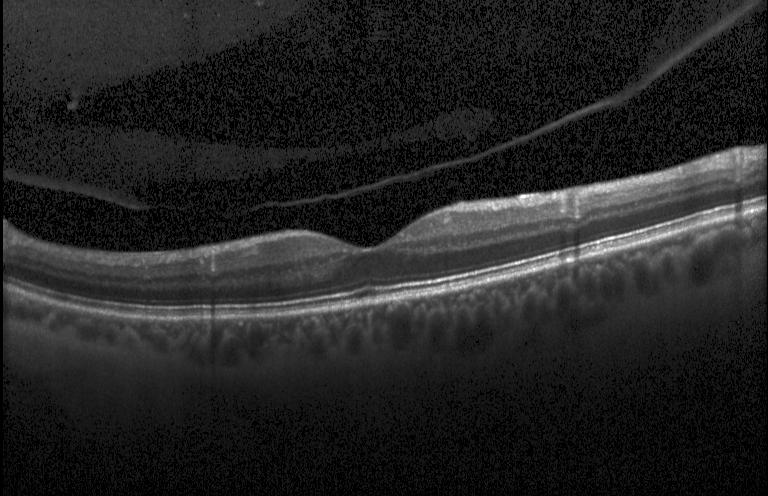

OCT B-scan; instrument: Heidelberg Spectralis; spectral-domain OCT
No choroidal neovascularization, diabetic macular edema, or drusen.